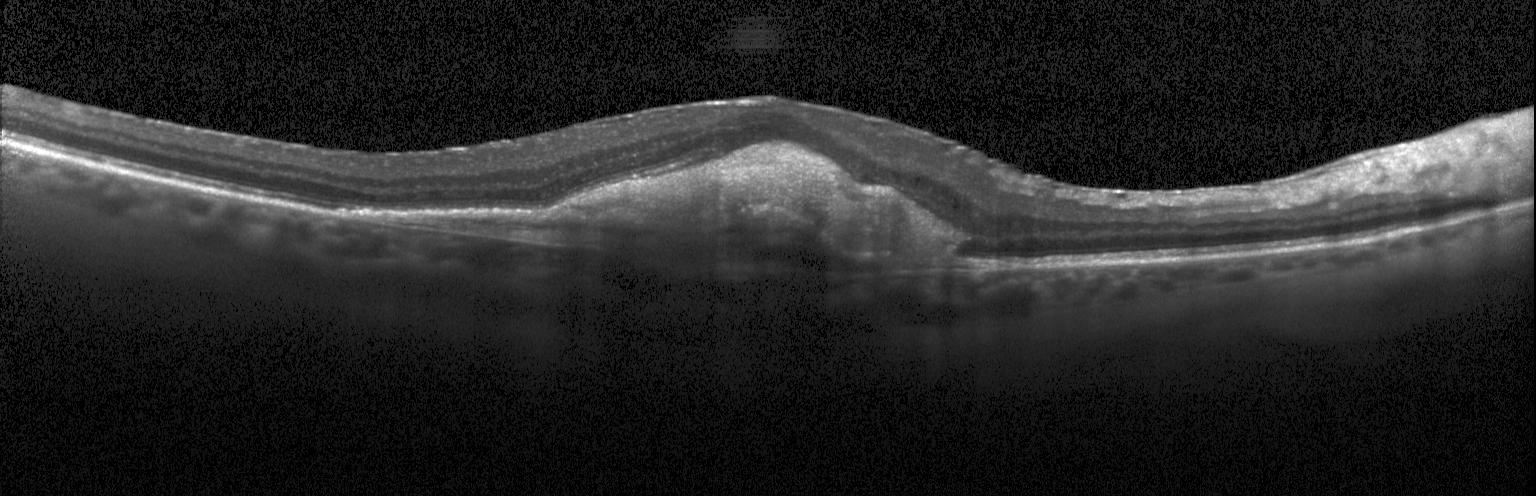 Impression: a choroidal neovascular membrane.